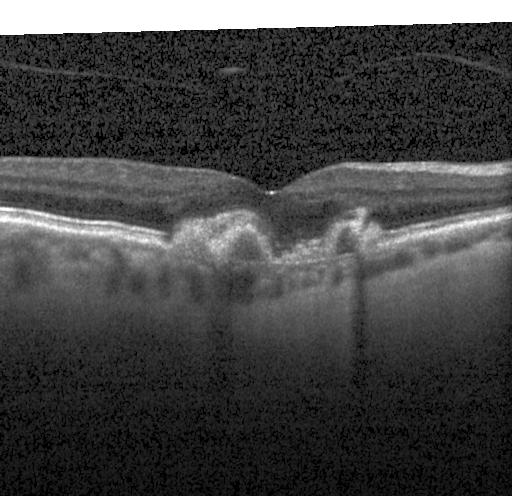

OCT finding: a choroidal neovascular membrane.